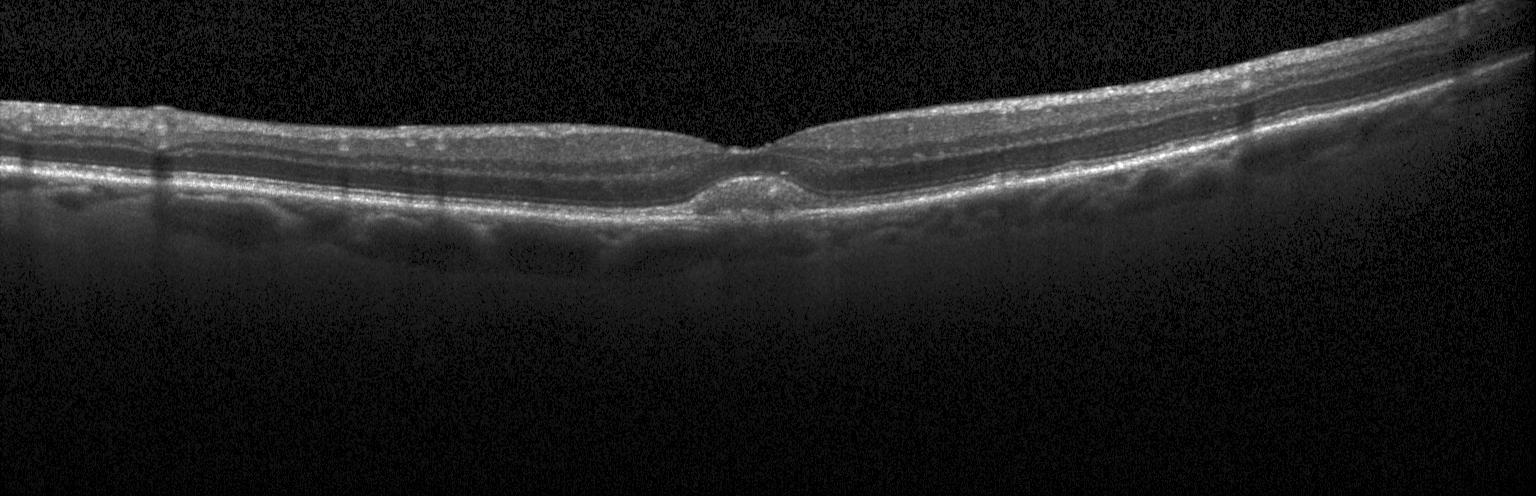 Assessment: a choroidal neovascular membrane.